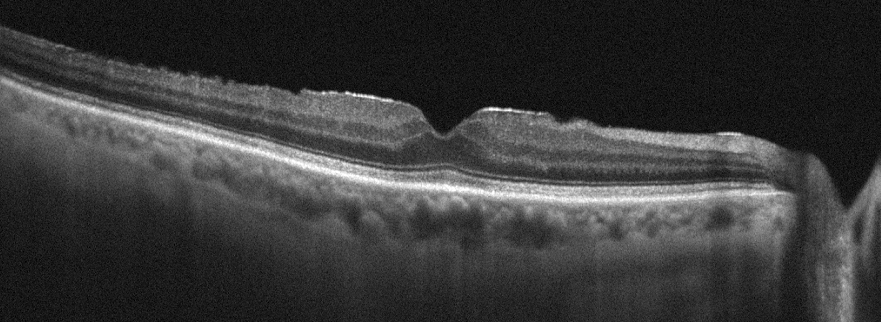

Impression: ERM.